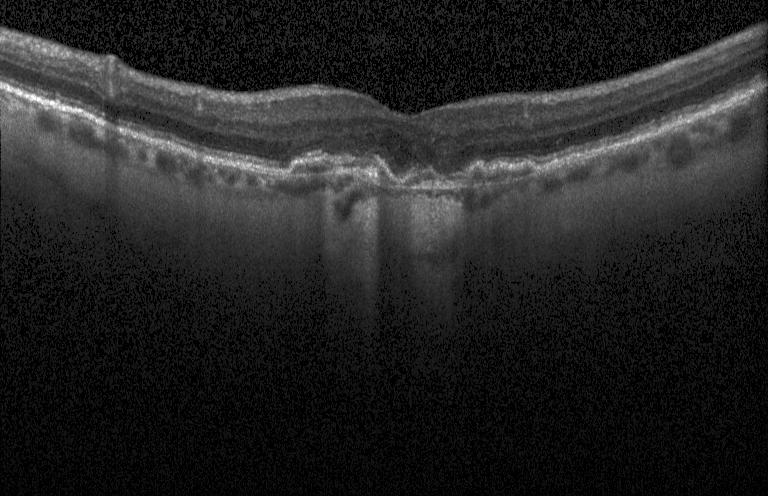
OCT line scan; macular scan — Impression: a choroidal neovascular membrane.